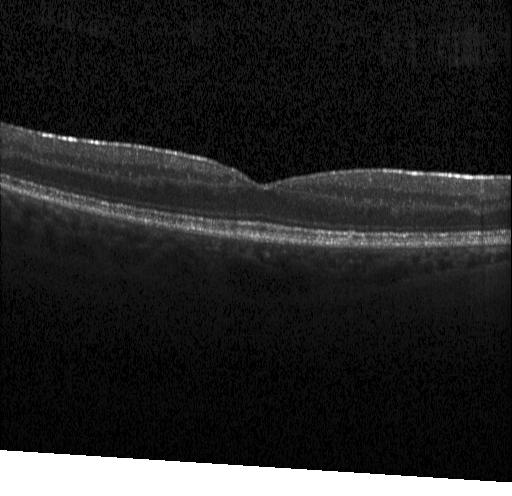 Acquired on a Heidelberg Spectralis. SD-OCT. Retinal OCT cross-section. Neither choroidal neovascularization, diabetic macular edema, nor drusen.